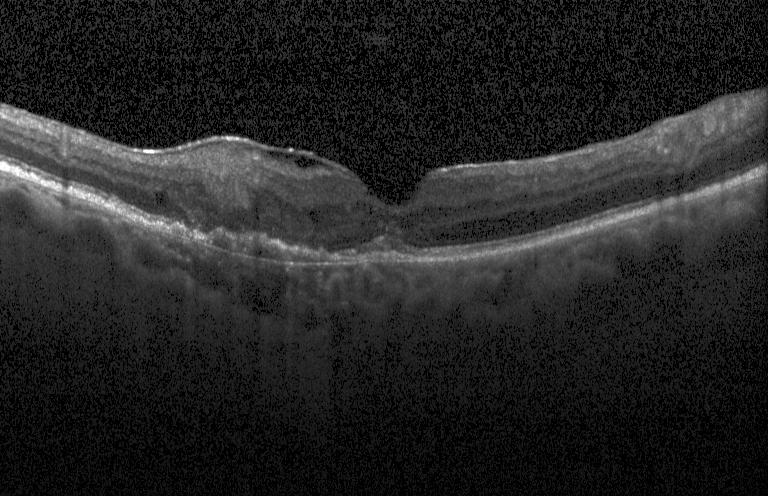 Retinal OCT B-scan; Heidelberg Spectralis OCT system; centered on the fovea; spectral-domain OCT
The scan shows a choroidal neovascular membrane.